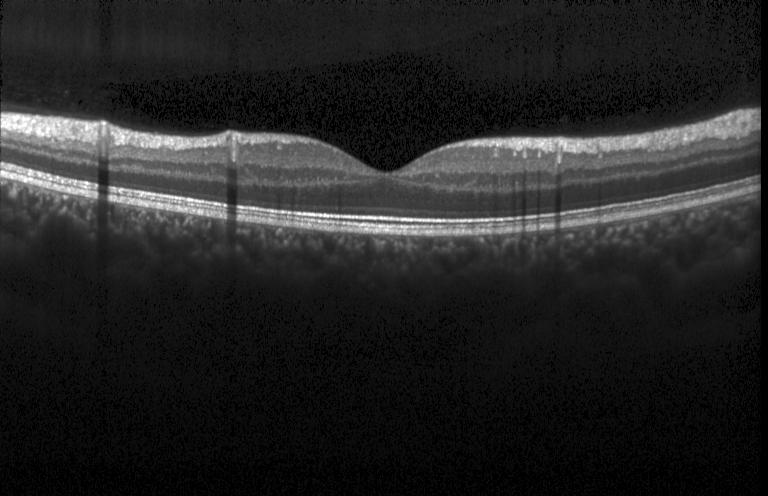 Assessment: no choroidal neovascularization, no diabetic macular edema, and no drusen.